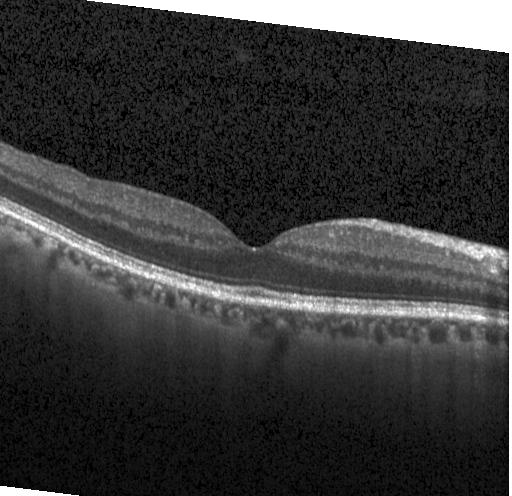 Diagnosis: neither choroidal neovascularization, diabetic macular edema, nor drusen.